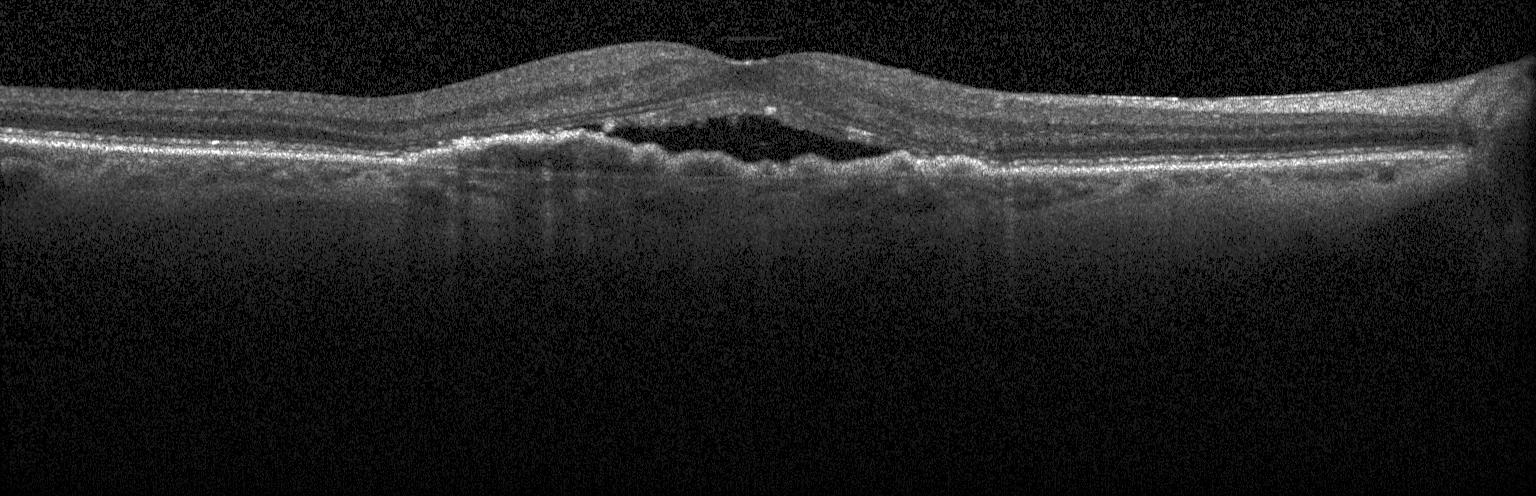 OCT B-scan showing choroidal neovascularization (CNV).